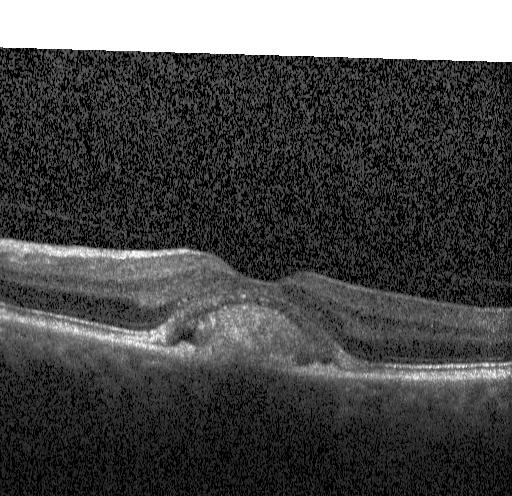 Optical coherence tomography scan; spectral-domain OCT; through the macula; Heidelberg Spectralis — Finding: a choroidal neovascular membrane.